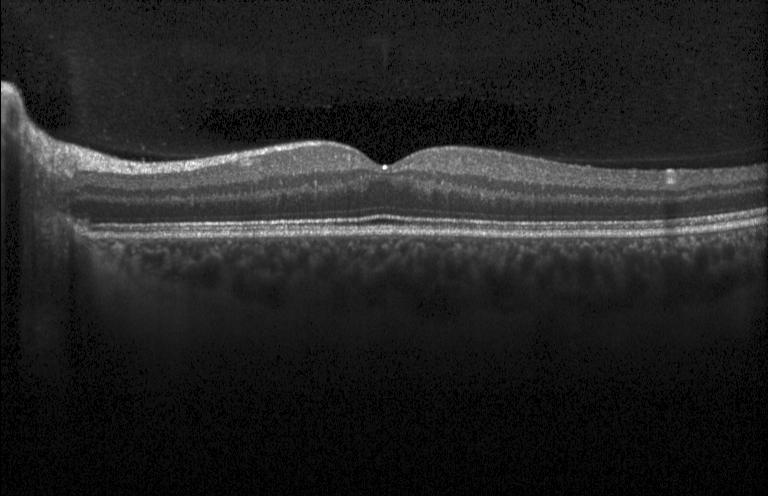 Retinal OCT cross-section showing neither choroidal neovascularization, diabetic macular edema, nor drusen.